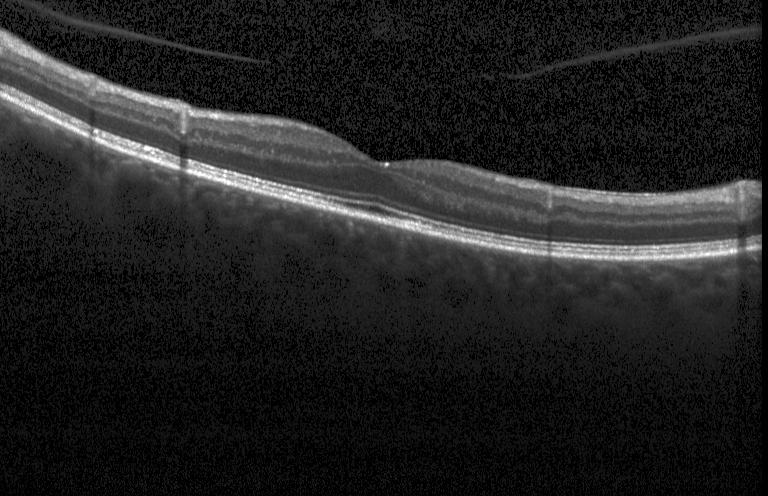
Optical coherence tomography B-scan; acquired on a Heidelberg Spectralis; centered on the fovea
Diagnosis: no choroidal neovascularization, diabetic macular edema, or drusen.